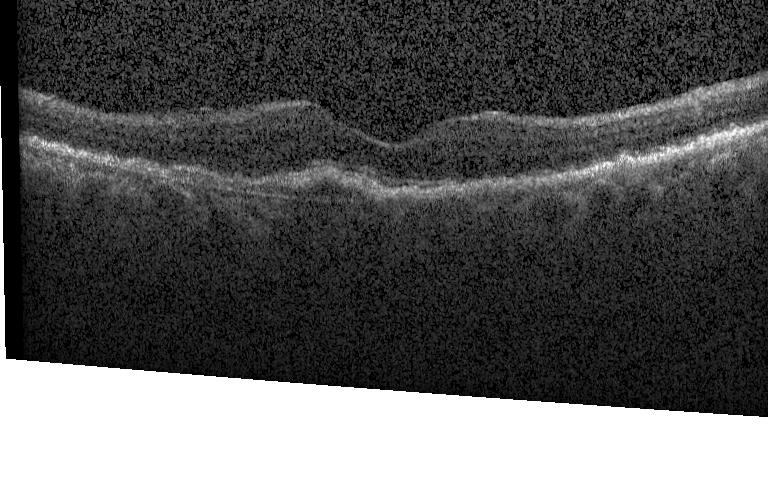

Optical coherence tomography scan. Assessment: CNV.